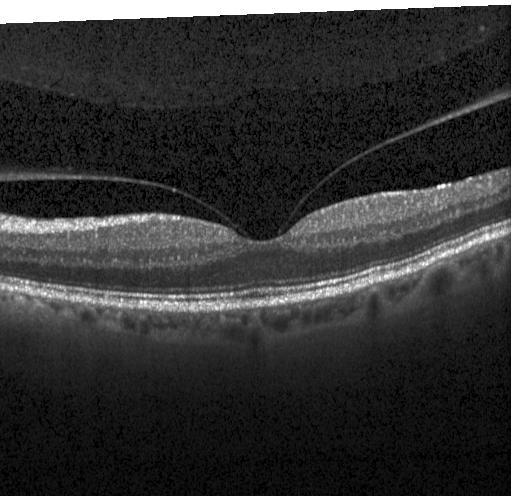

Finding: neither choroidal neovascularization, diabetic macular edema, nor drusen.